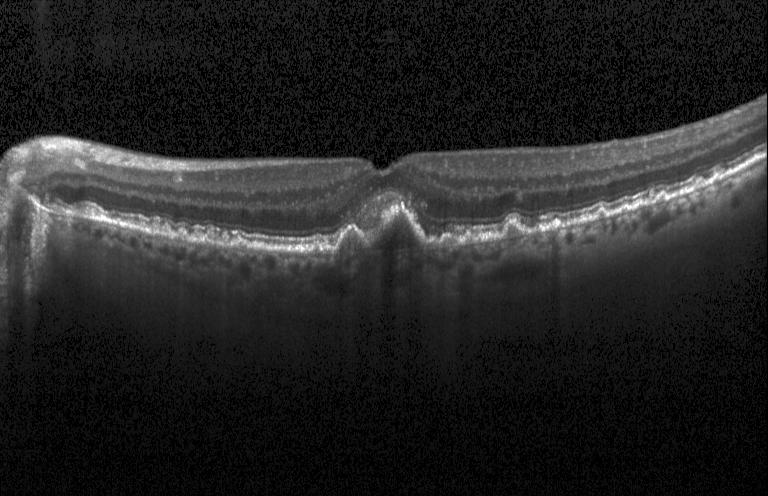

SD-OCT, optical coherence tomography B-scan, acquired on a Heidelberg Spectralis, through the macula. Finding: CNV.